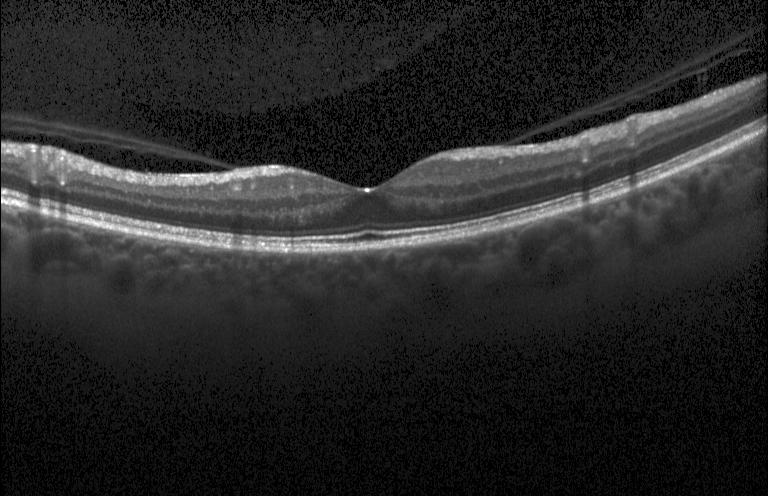
Retinal OCT B-scan
This B-scan demonstrates no choroidal neovascularization, no diabetic macular edema, and no drusen.